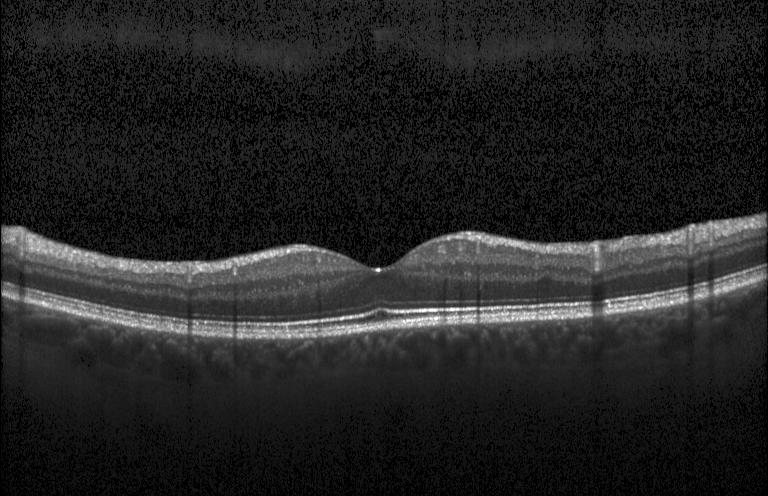
Fovea-centered. Spectral-domain optical coherence tomography. Retinal OCT cross-section. Heidelberg Spectralis OCT system — Assessment: no evidence of choroidal neovascularization, diabetic macular edema, or drusen.